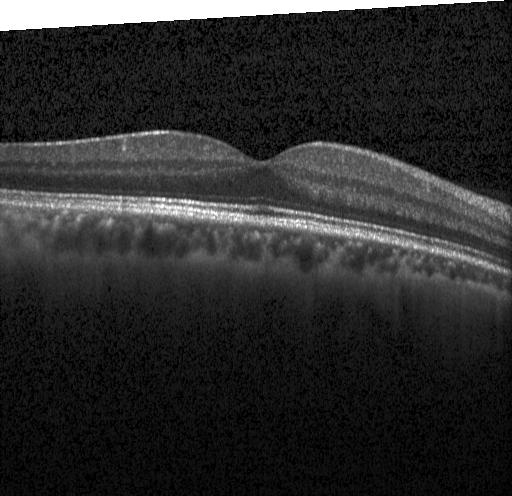
Optical coherence tomography B-scan · instrument: Heidelberg Spectralis.
Finding: no evidence of CNV, DME, or drusen.